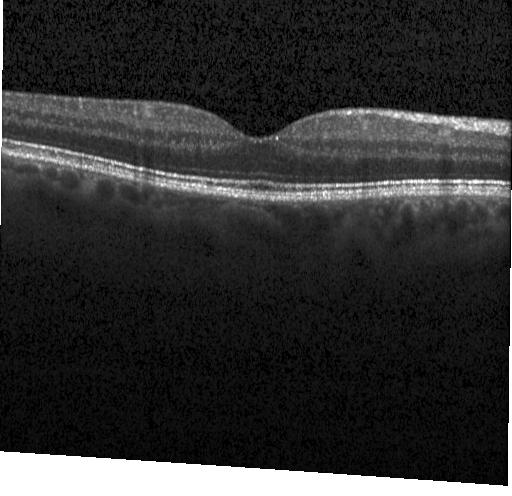

Optical coherence tomography scan
Diagnosis: no choroidal neovascularization, diabetic macular edema, or drusen.